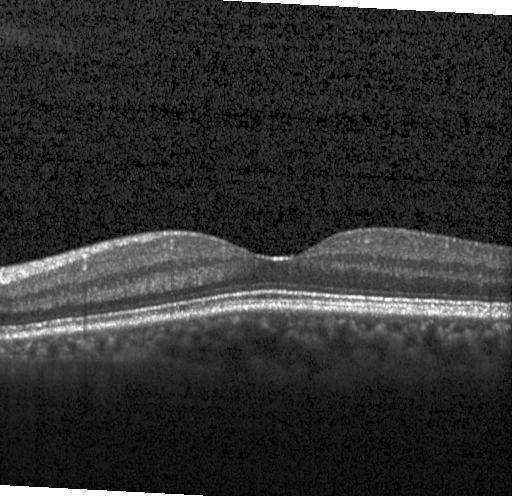

Spectral-domain OCT; macular scan; optical coherence tomography B-scan; Heidelberg Spectralis OCT system — Dx: no CNV, no DME, and no drusen.